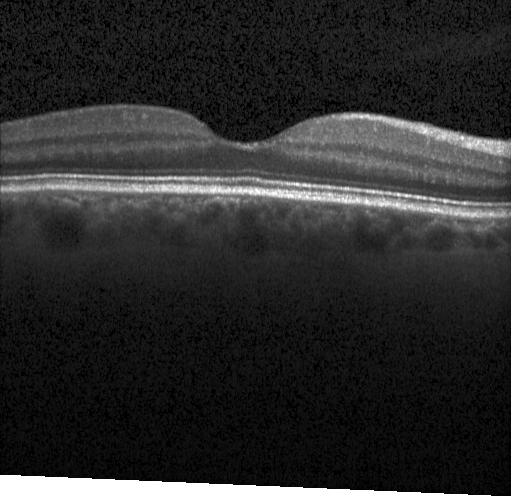

OCT B-scan. Spectral-domain OCT. Horizontal scan through the fovea
No evidence of CNV, DME, or drusen.